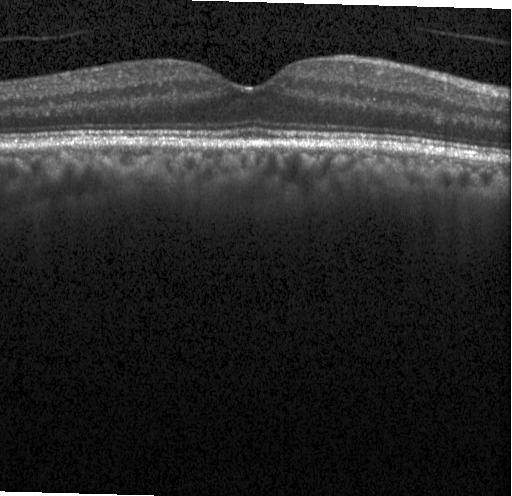

This B-scan demonstrates neither choroidal neovascularization, diabetic macular edema, nor drusen.